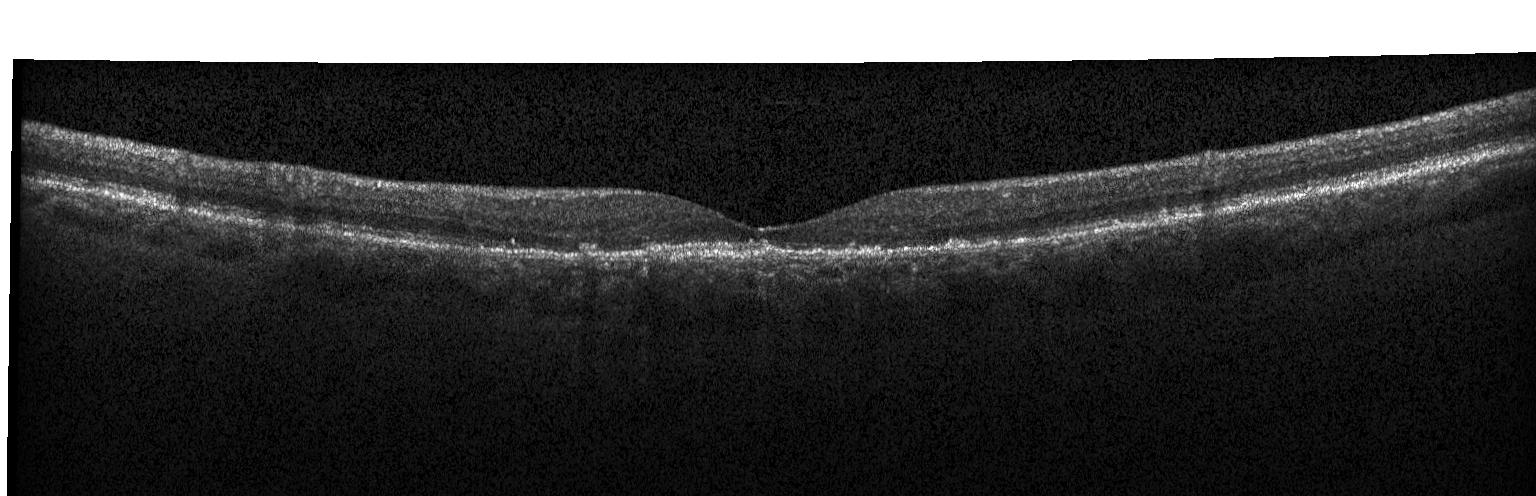

Centered on the fovea, retinal OCT B-scan.
Dx: a choroidal neovascular membrane.